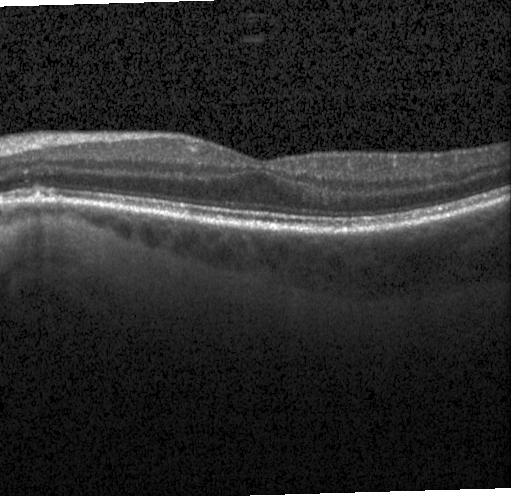
Retinal OCT cross-section showing multiple drusen.